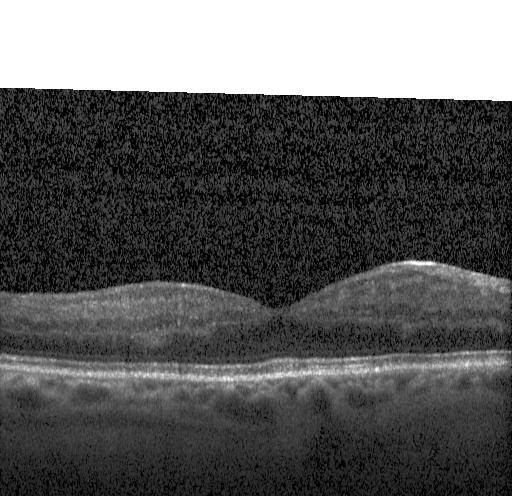
OCT B-scan showing no evidence of choroidal neovascularization, diabetic macular edema, or drusen.